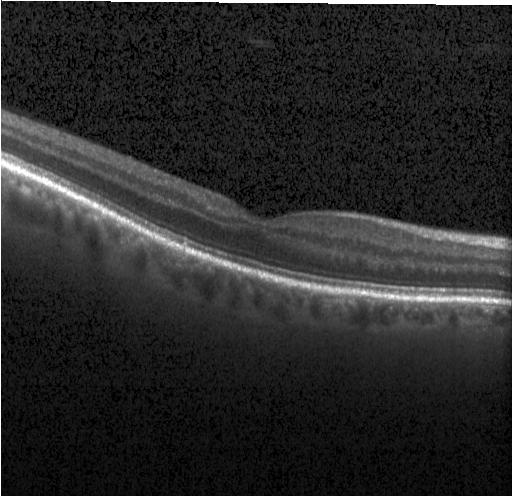

Finding: neither choroidal neovascularization, diabetic macular edema, nor drusen.